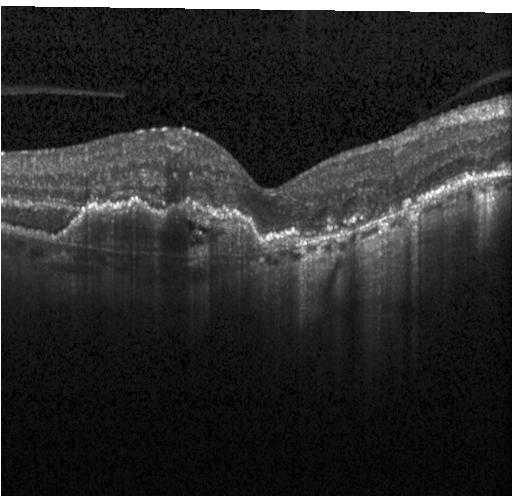
Retinal OCT cross-section
Diagnosis: choroidal neovascularization.